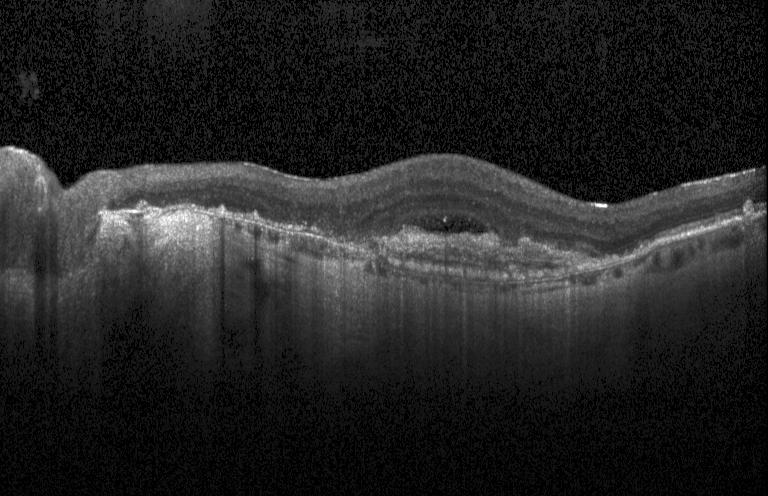 Spectral-domain optical coherence tomography; Heidelberg Spectralis OCT system; OCT line scan.
Impression: CNV.